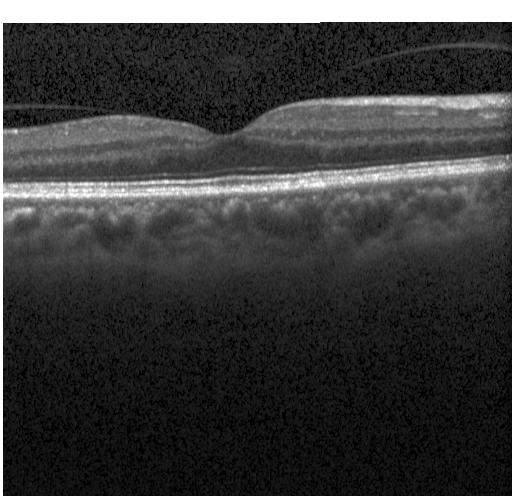

Diagnosis: no evidence of CNV, DME, or drusen.